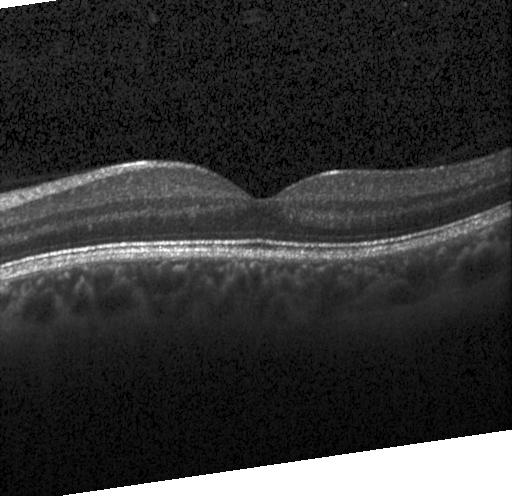 Retinal OCT cross-section; fovea-centered
Dx: no choroidal neovascularization, no diabetic macular edema, and no drusen.